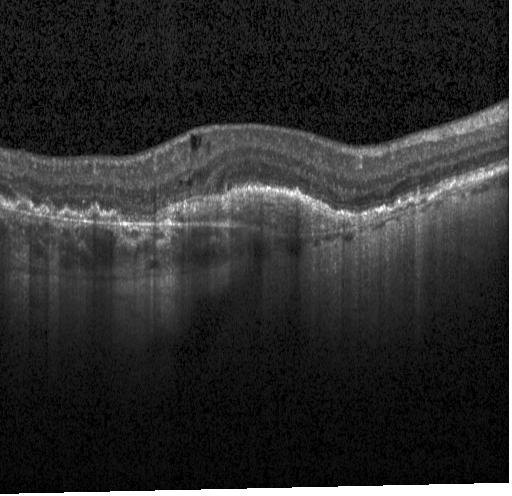
Impression: a choroidal neovascular membrane.